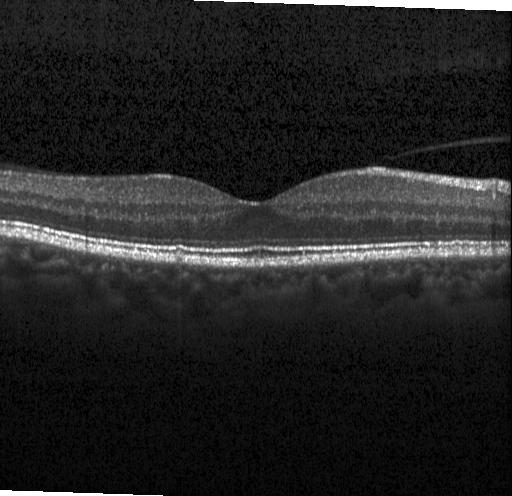 Retinal OCT cross-section. Macular scan
Impression: no evidence of choroidal neovascularization, diabetic macular edema, or drusen.